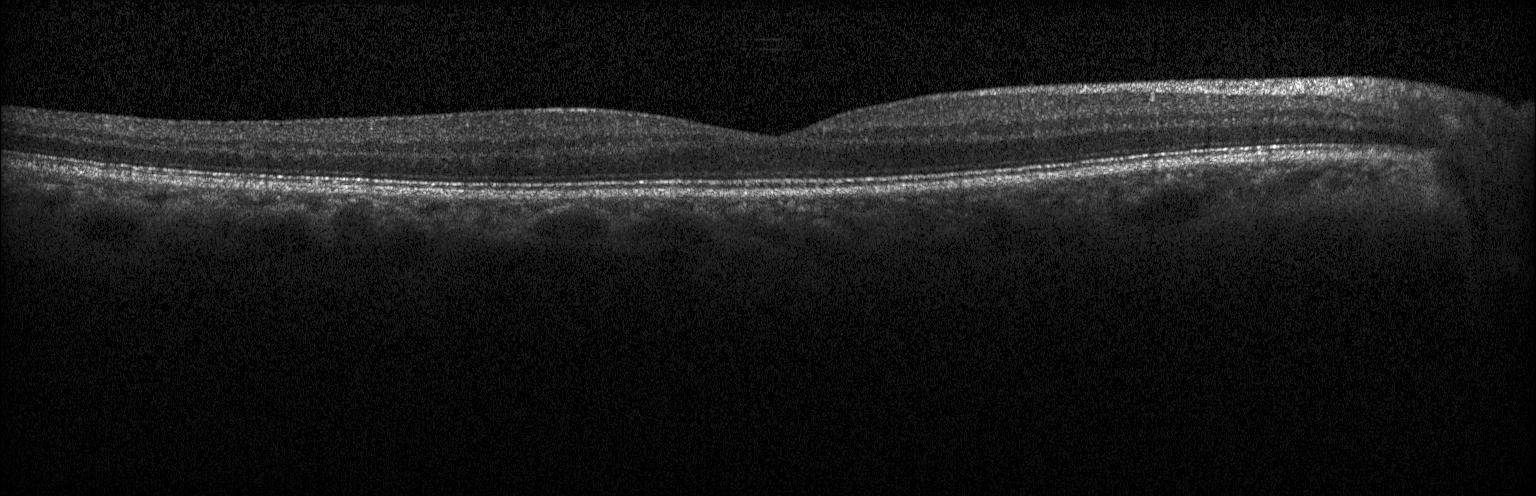
Impression: no evidence of choroidal neovascularization, diabetic macular edema, or drusen.